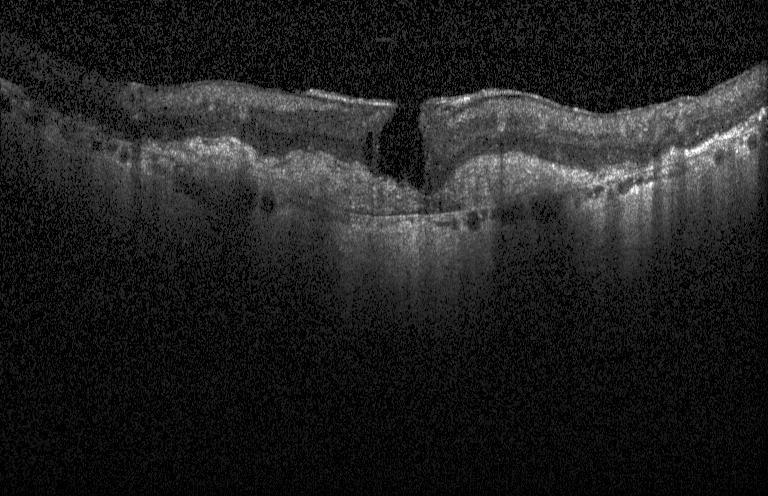
OCT line scan; Heidelberg Spectralis OCT system.
Dx: a choroidal neovascular membrane.